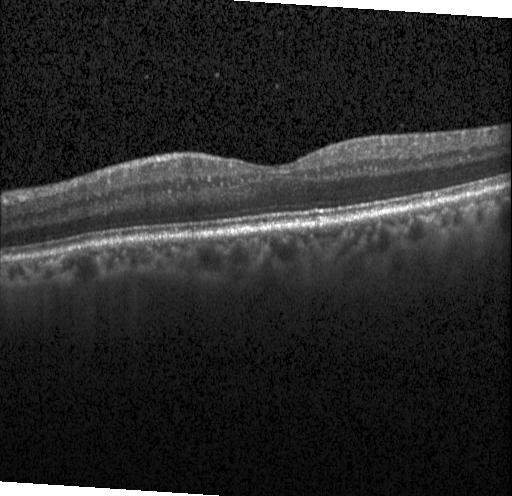
Retinal OCT B-scan
Finding: no evidence of CNV, DME, or drusen.